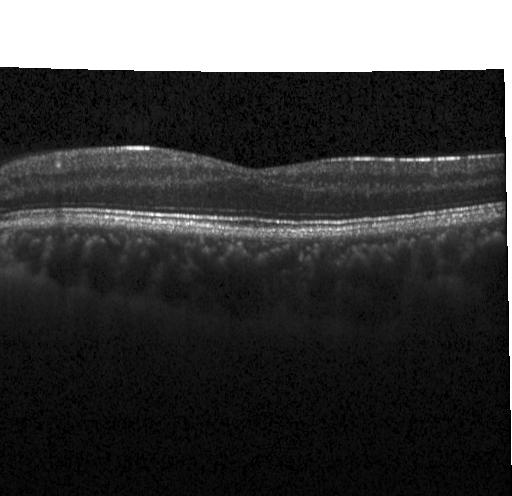
OCT B-scan.
Macular OCT: no evidence of choroidal neovascularization, diabetic macular edema, or drusen.